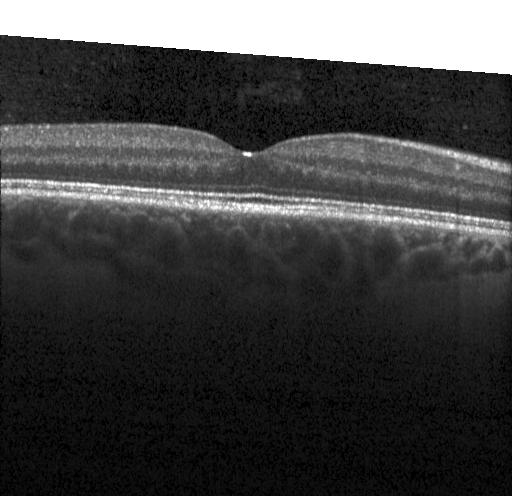 Retinal OCT cross-section · SD-OCT. The scan shows neither choroidal neovascularization, diabetic macular edema, nor drusen.